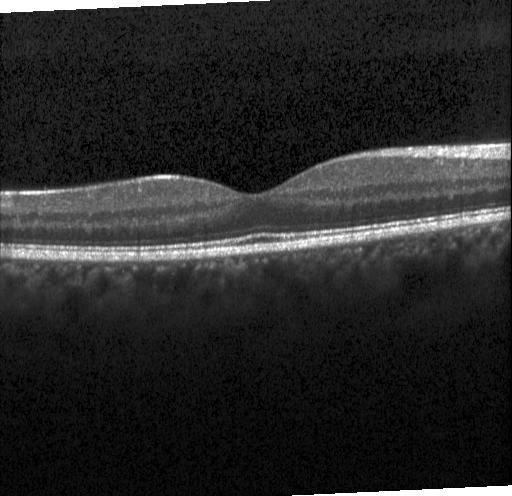 Finding: no evidence of choroidal neovascularization, diabetic macular edema, or drusen.